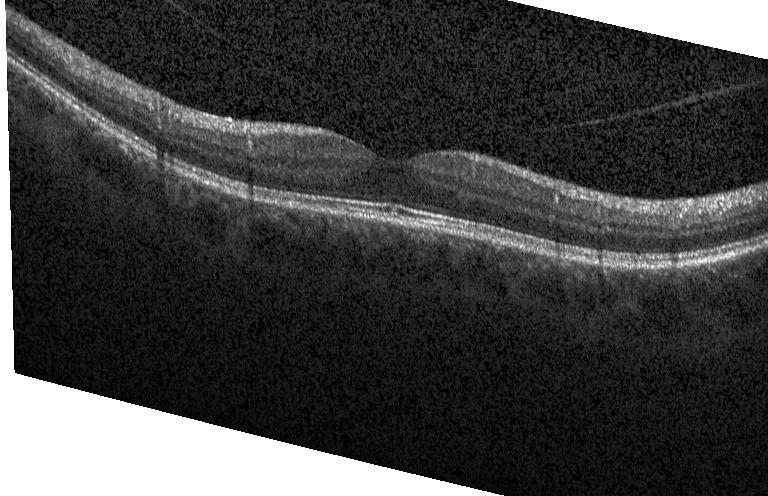
Diagnosis: no CNV, no DME, and no drusen.